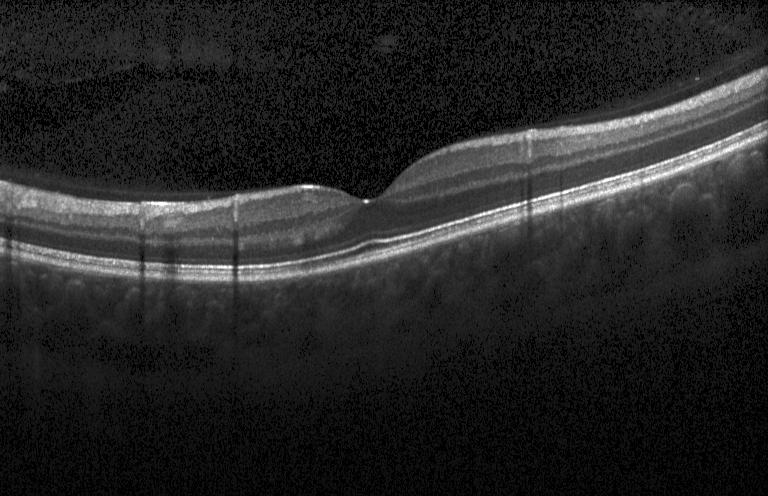 Optical coherence tomography B-scan, SD-OCT, Heidelberg Spectralis, through the macula. Impression: no evidence of choroidal neovascularization, diabetic macular edema, or drusen.